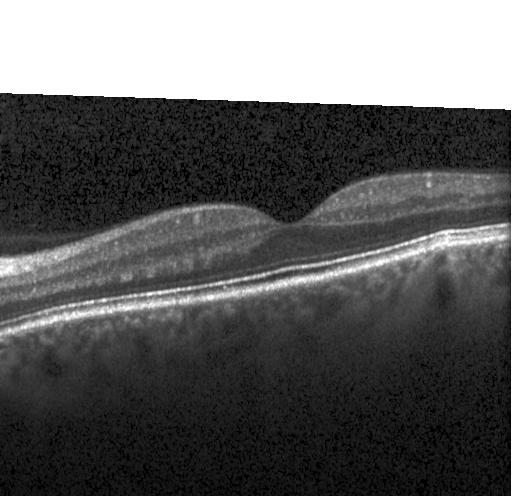 Centered on the fovea · spectral-domain optical coherence tomography · OCT line scan. Finding: neither choroidal neovascularization, diabetic macular edema, nor drusen.